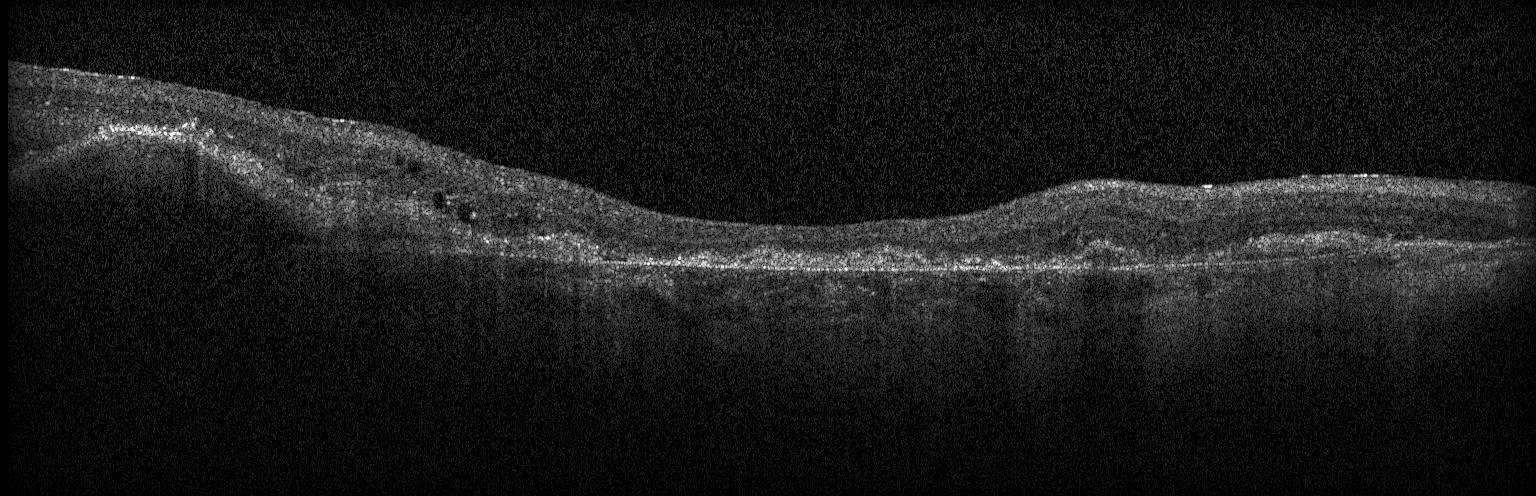
SD-OCT, instrument: Heidelberg Spectralis, optical coherence tomography B-scan
Diagnosis: choroidal neovascularization (CNV).